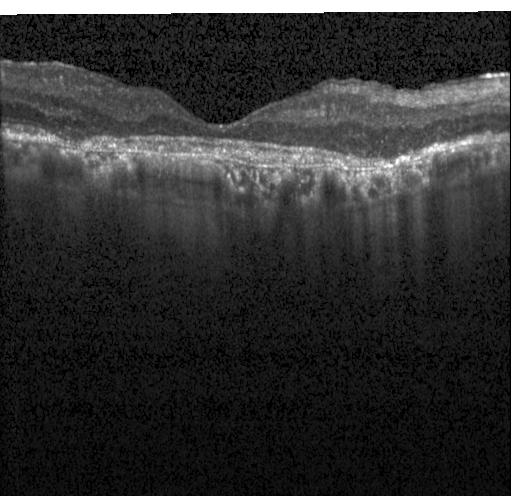
Retinal OCT cross-section. Heidelberg Spectralis
A choroidal neovascular membrane.